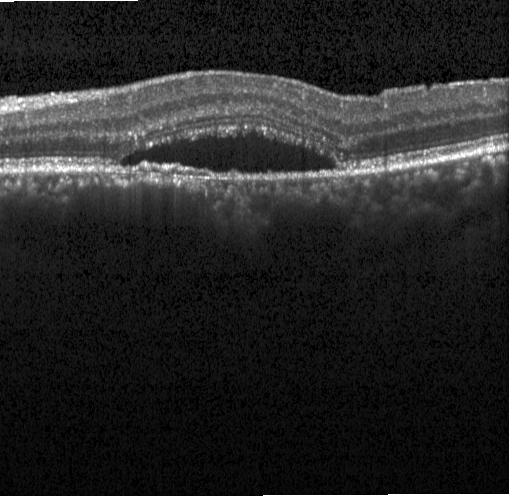
Assessment: a choroidal neovascular membrane.